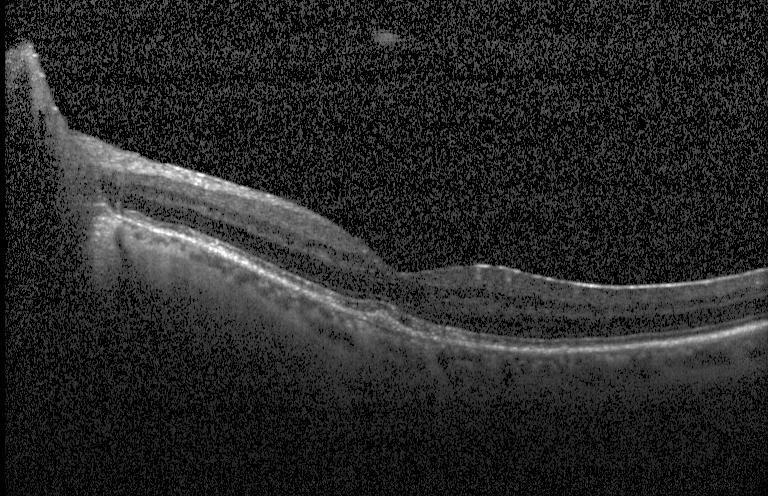

Horizontal scan through the fovea · instrument: Heidelberg Spectralis · spectral-domain optical coherence tomography · OCT B-scan — Dx: a choroidal neovascular membrane.